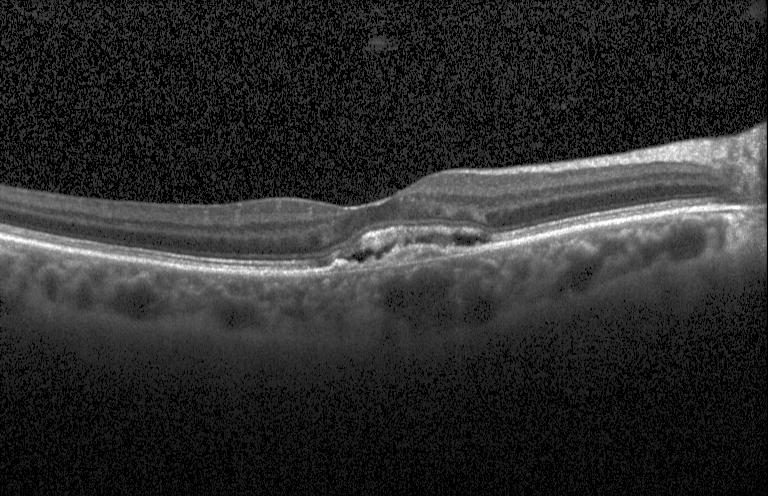 Macular scan; instrument: Heidelberg Spectralis; retinal OCT cross-section; spectral-domain optical coherence tomography — Dx: a choroidal neovascular membrane.